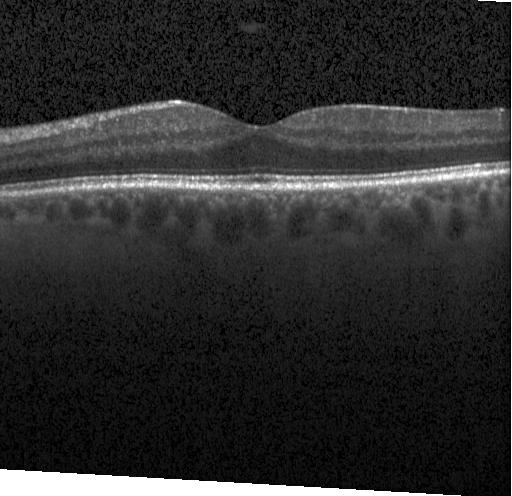

Spectral-domain OCT B-scan: no choroidal neovascularization, diabetic macular edema, or drusen.